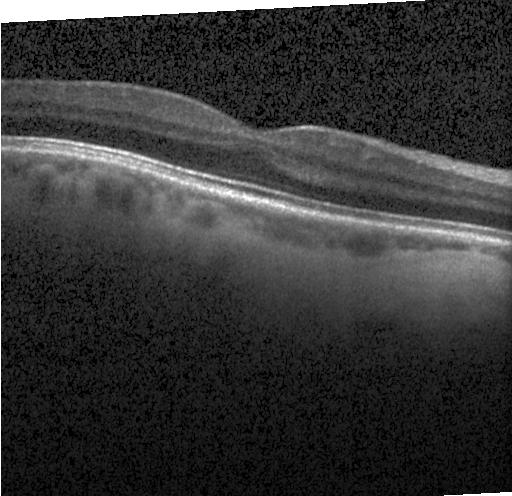

Diagnosis: no evidence of choroidal neovascularization, diabetic macular edema, or drusen.